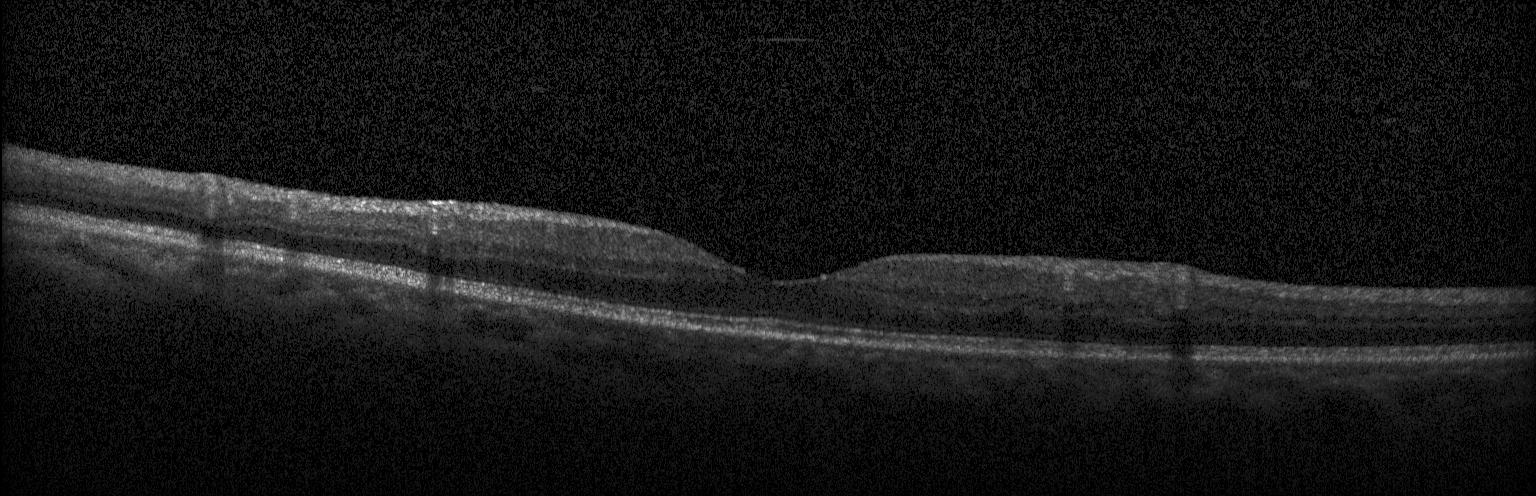

Macular scan; OCT B-scan; SD-OCT; instrument: Heidelberg Spectralis. Impression: no choroidal neovascularization, no diabetic macular edema, and no drusen.